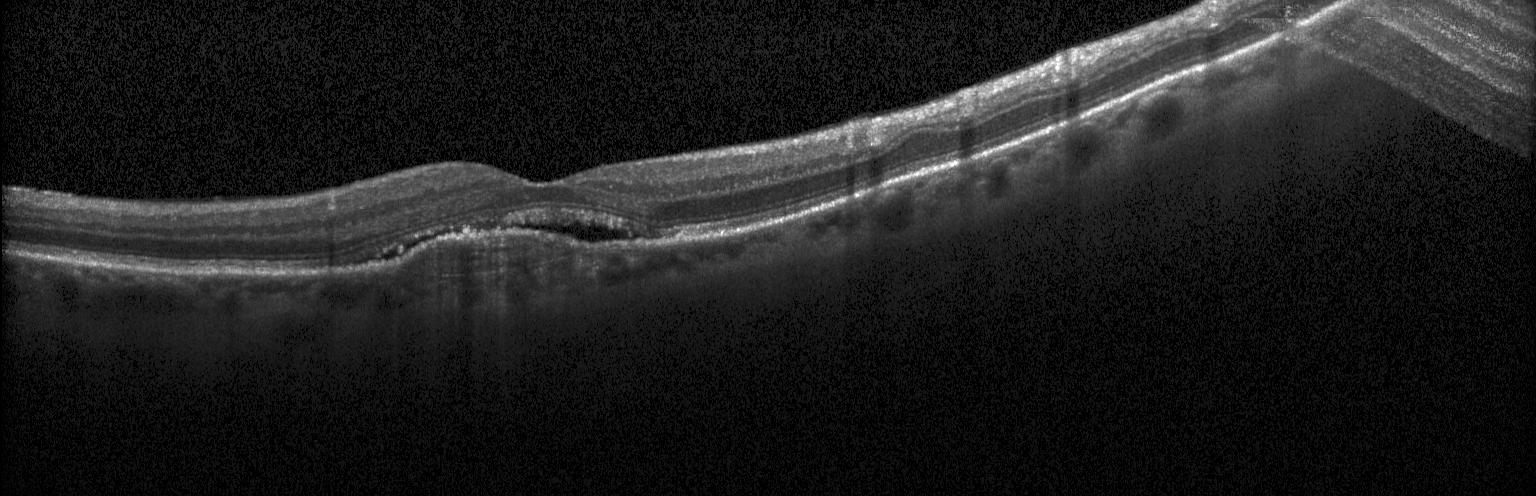 OCT line scan. Finding: choroidal neovascularization.